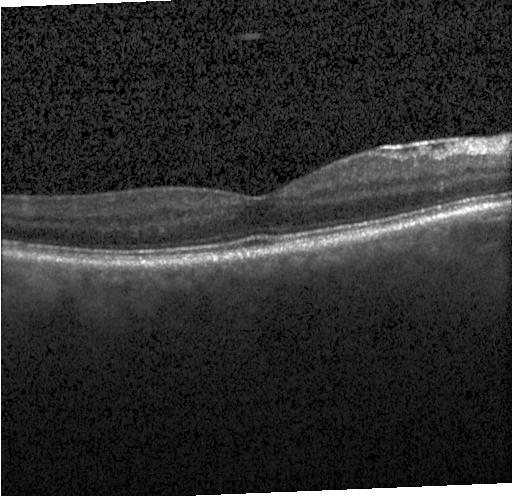 Optical coherence tomography B-scan · SD-OCT · horizontal scan through the fovea. Diagnosis: no choroidal neovascularization, no diabetic macular edema, and no drusen.